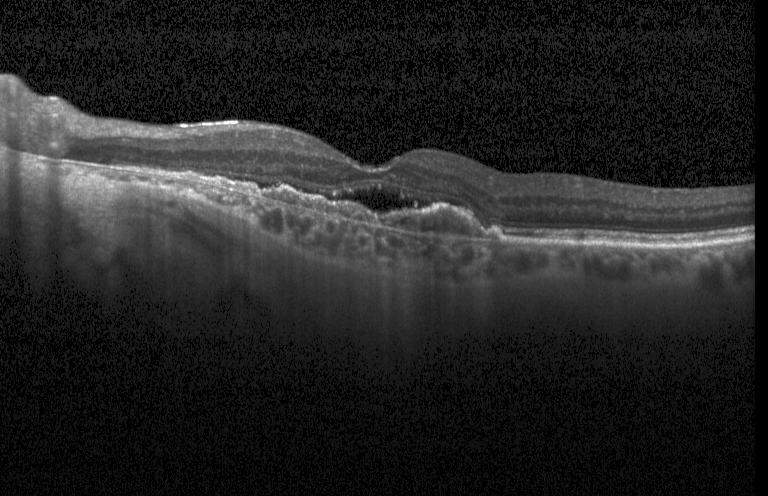

OCT line scan, spectral-domain optical coherence tomography, through the macula, Heidelberg Spectralis OCT system — Impression: choroidal neovascularization.